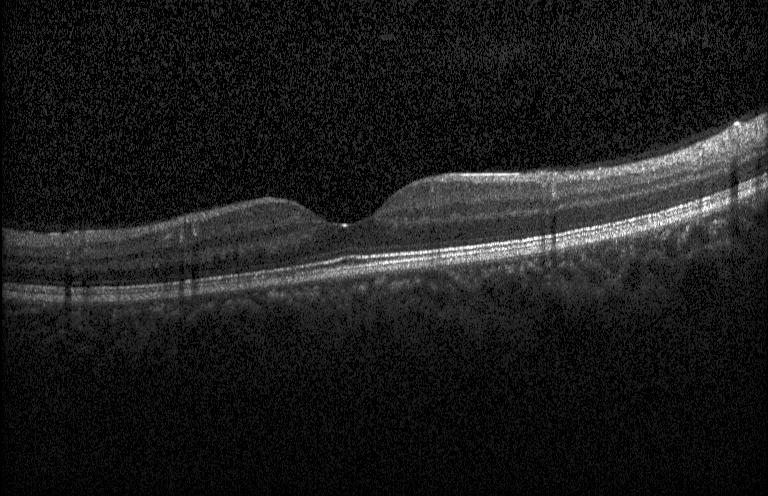

Optical coherence tomography B-scan.
Dx: no evidence of CNV, DME, or drusen.